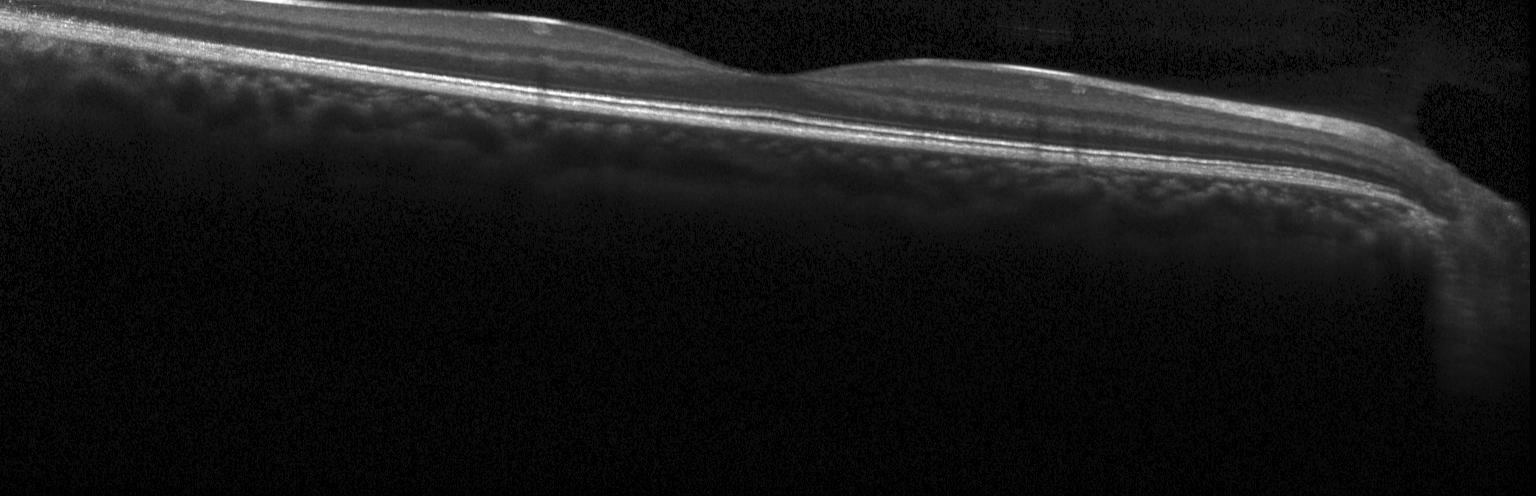

Retinal OCT cross-section. Spectral-domain OCT. Acquired on a Heidelberg Spectralis. Centered on the fovea. Diagnosis: no CNV, no DME, and no drusen.